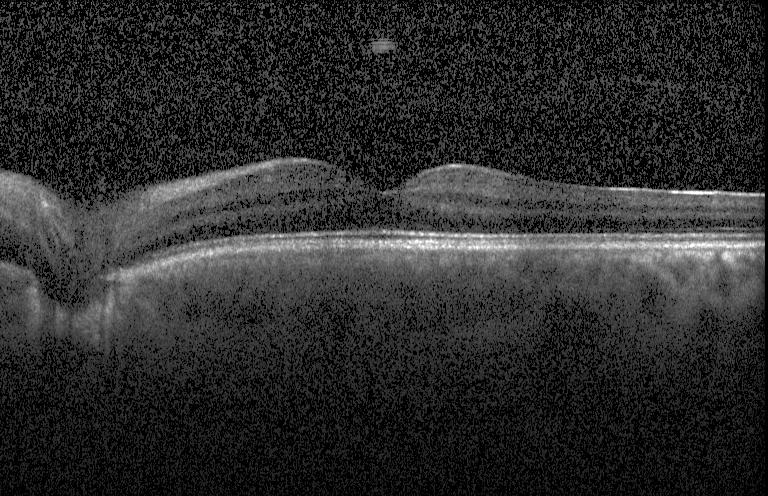
Retinal OCT cross-section; spectral-domain OCT; acquired on a Heidelberg Spectralis — Dx: no choroidal neovascularization, diabetic macular edema, or drusen.